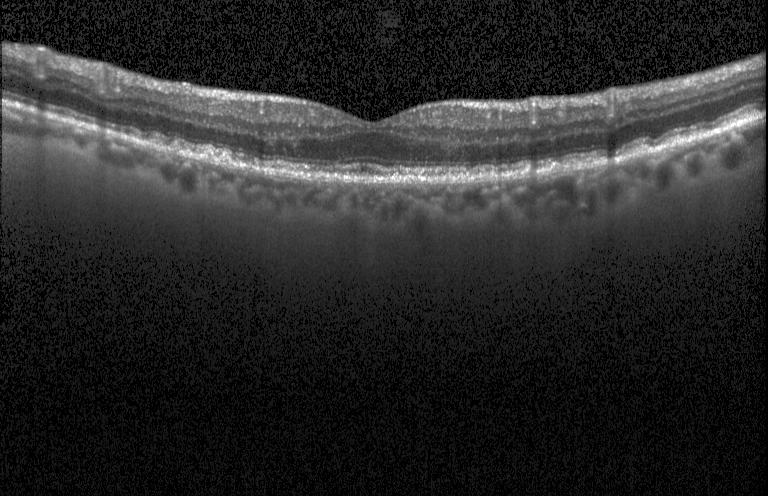
Heidelberg Spectralis OCT system; optical coherence tomography B-scan — Impression: sub-RPE drusenoid deposits.